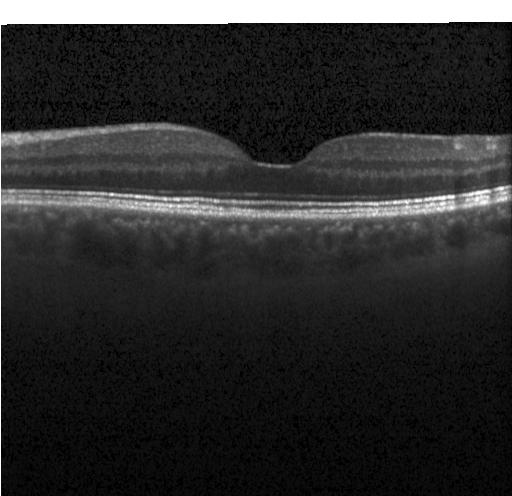 Retinal OCT B-scan; Heidelberg Spectralis OCT system; macular scan; spectral-domain optical coherence tomography
Dx: neither CNV, DME, nor drusen.